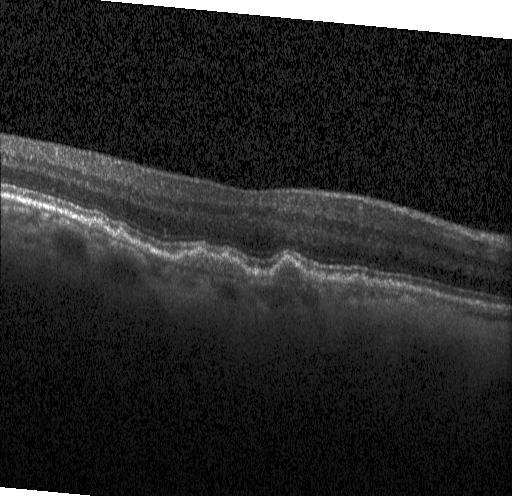

Heidelberg Spectralis OCT system. Spectral-domain OCT. Centered on the fovea. Optical coherence tomography B-scan — Finding: sub-RPE drusenoid deposits.